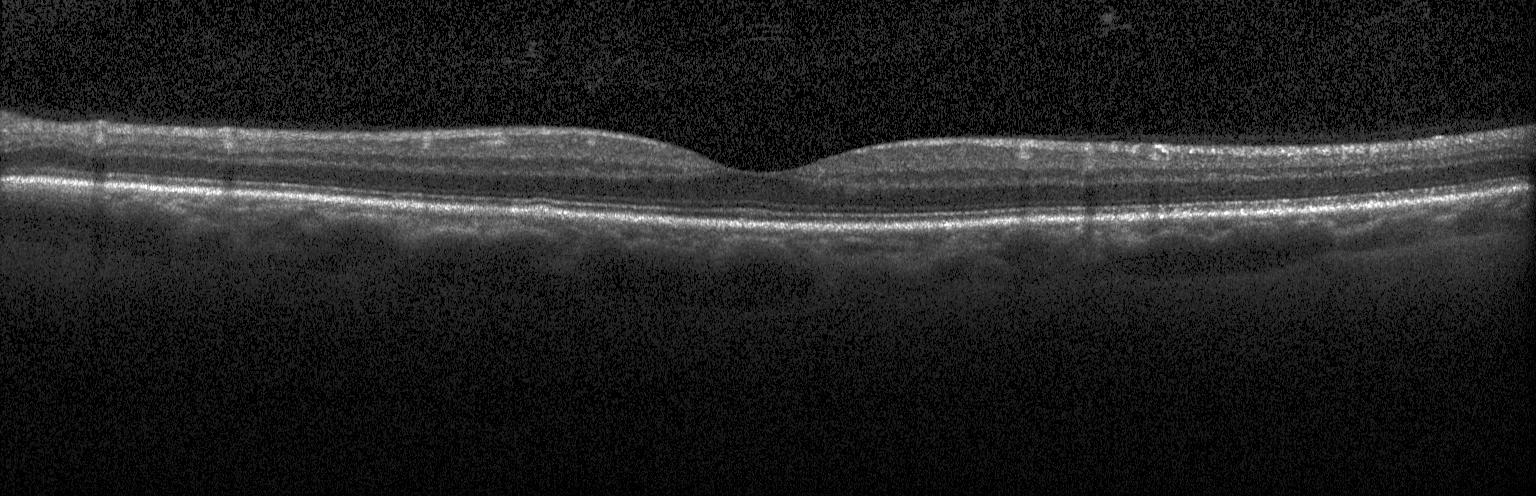

OCT scan showing no choroidal neovascularization, no diabetic macular edema, and no drusen.